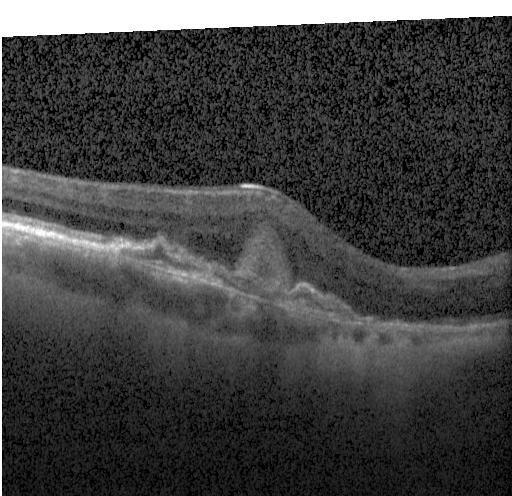

Finding: a choroidal neovascular membrane.